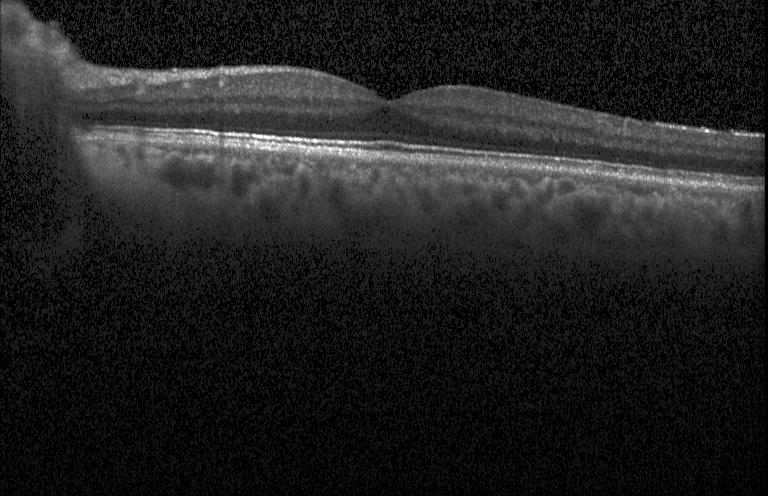
Centered on the fovea. Spectral-domain optical coherence tomography. Retinal OCT cross-section.
Dx: no evidence of choroidal neovascularization, diabetic macular edema, or drusen.